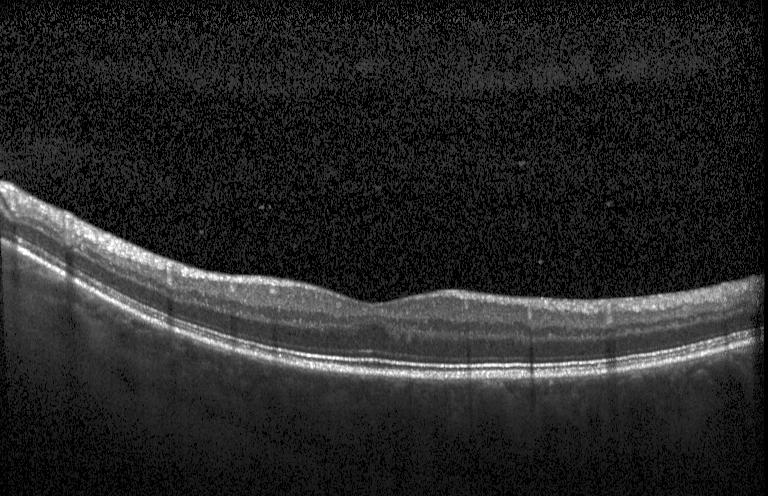
Diagnosis: neither CNV, DME, nor drusen.